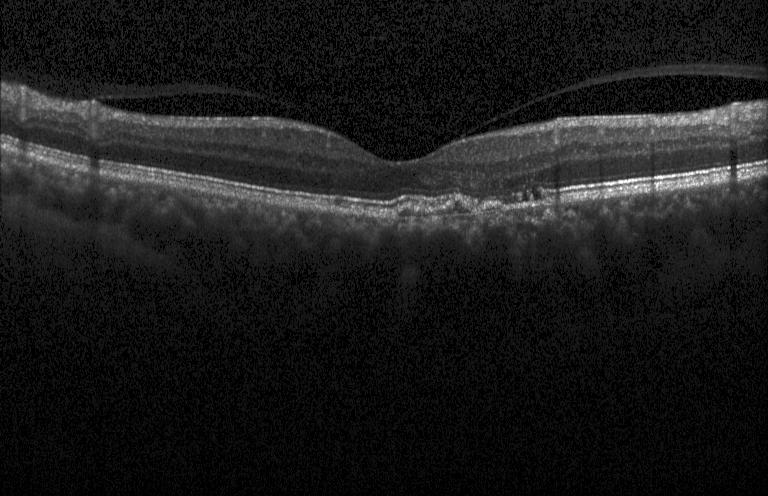 Heidelberg Spectralis OCT system, retinal OCT cross-section, fovea-centered. Finding: multiple drusen.